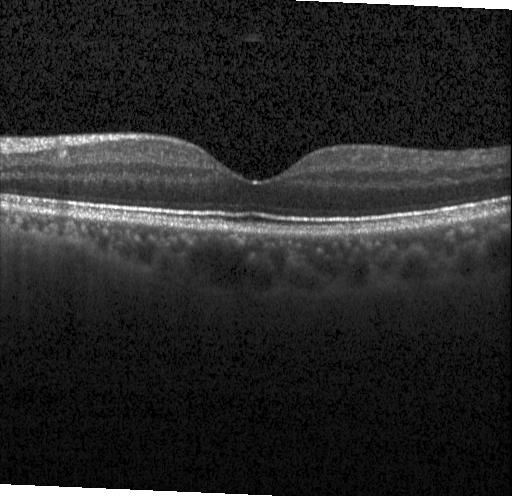 OCT line scan — Assessment: no evidence of CNV, DME, or drusen.